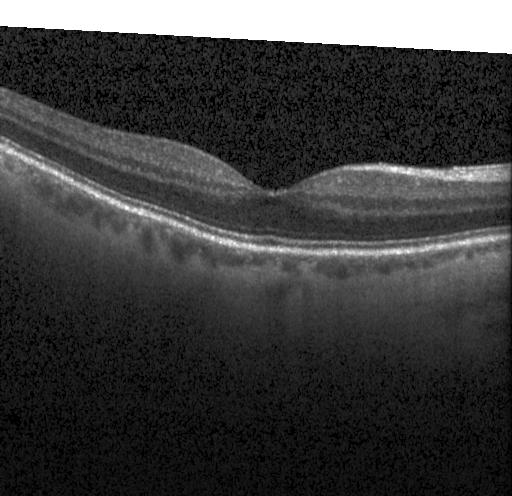
Impression: no CNV, no DME, and no drusen.